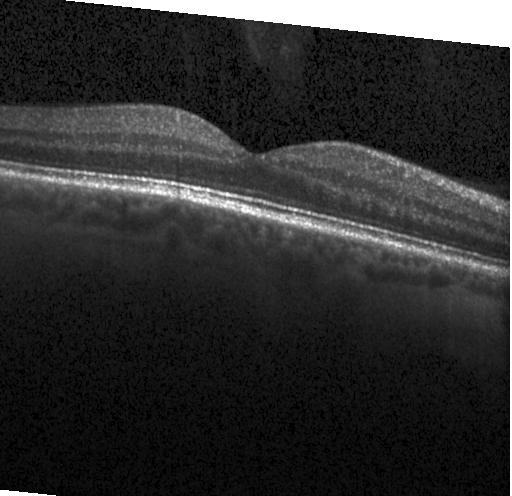 Heidelberg Spectralis. OCT B-scan. Dx: no evidence of choroidal neovascularization, diabetic macular edema, or drusen.